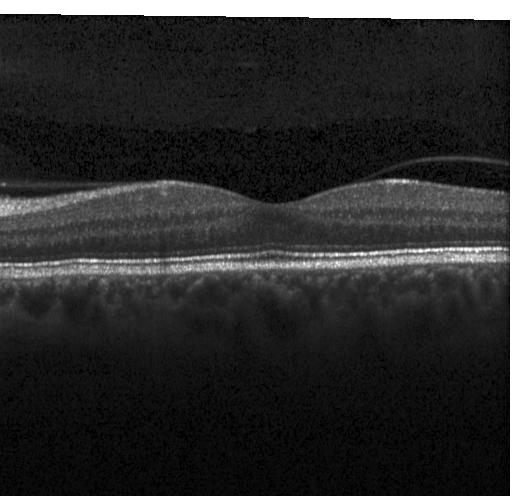
Dx: no evidence of choroidal neovascularization, diabetic macular edema, or drusen.